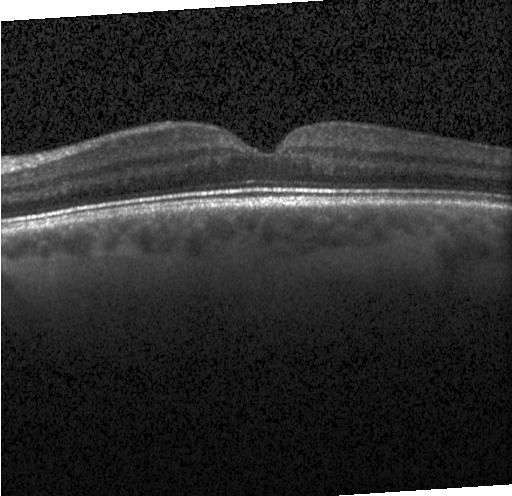 OCT B-scan showing no choroidal neovascularization, diabetic macular edema, or drusen.